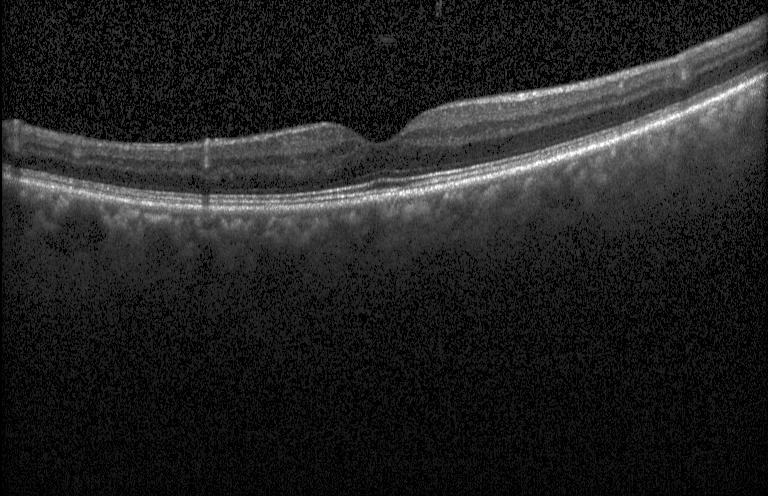 OCT B-scan.
Diagnosis: no evidence of choroidal neovascularization, diabetic macular edema, or drusen.